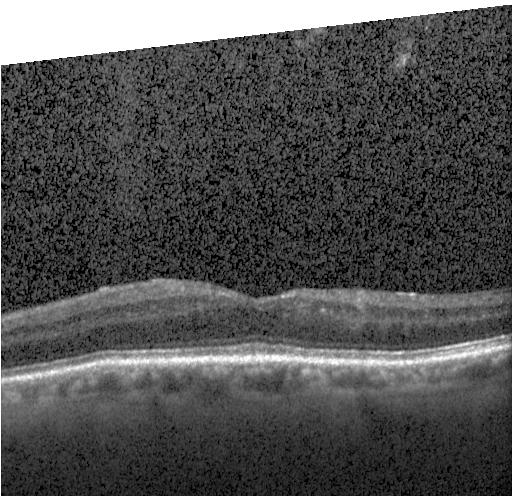

No evidence of CNV, DME, or drusen.